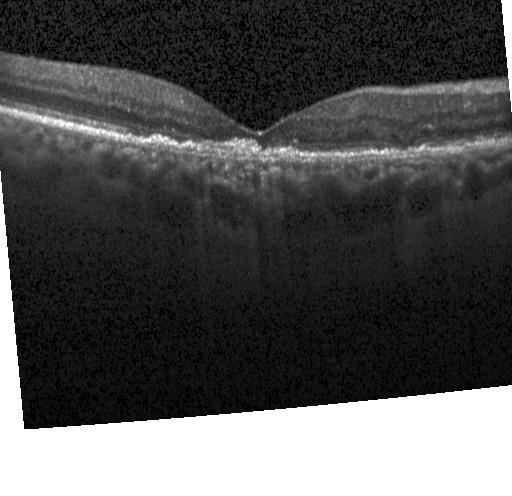
Macular OCT: a choroidal neovascular membrane.